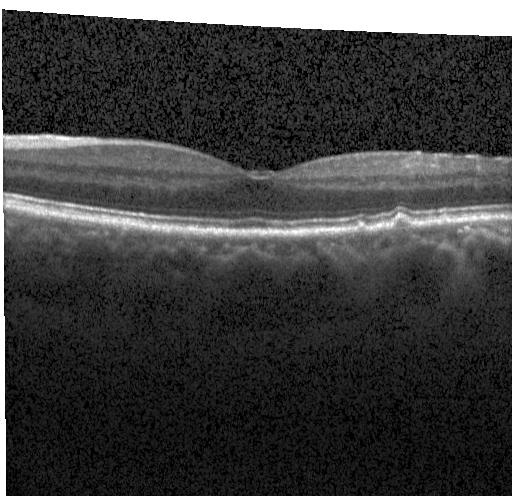

Macular OCT: multiple drusen.